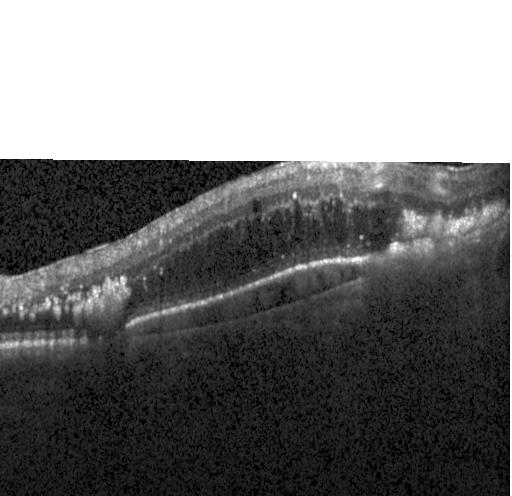

The scan shows diabetic macular edema (DME).